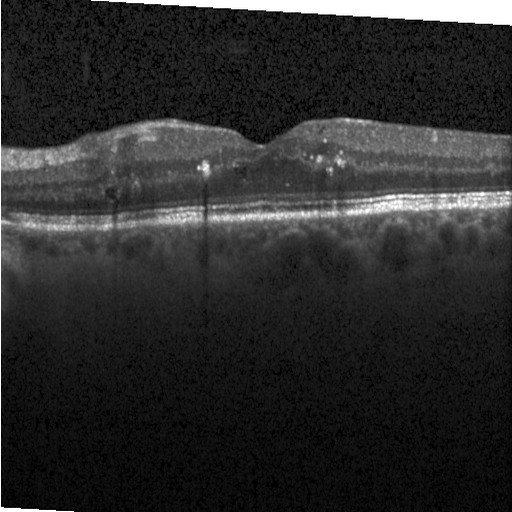

OCT B-scan, macular scan. Dx: diabetic macular edema.